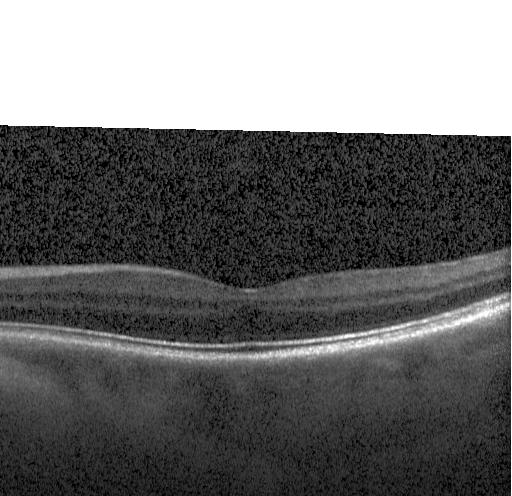

OCT B-scan.
Impression: no evidence of choroidal neovascularization, diabetic macular edema, or drusen.